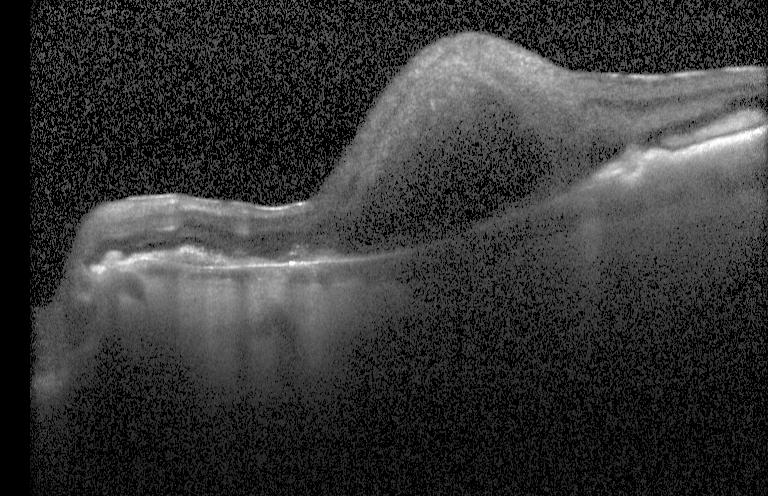

Through the macula; Heidelberg Spectralis OCT system; spectral-domain OCT; OCT B-scan.
Finding: a choroidal neovascular membrane.